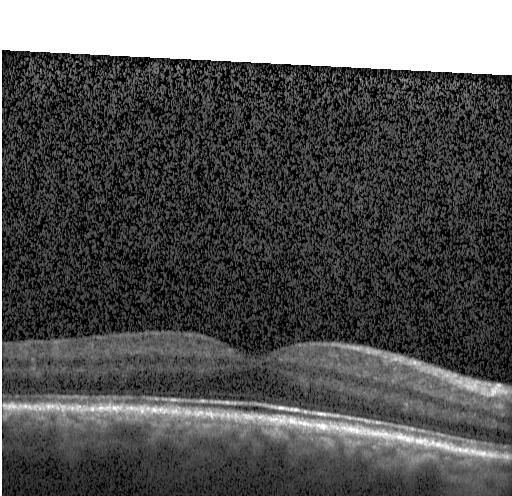
Finding: no evidence of choroidal neovascularization, diabetic macular edema, or drusen.